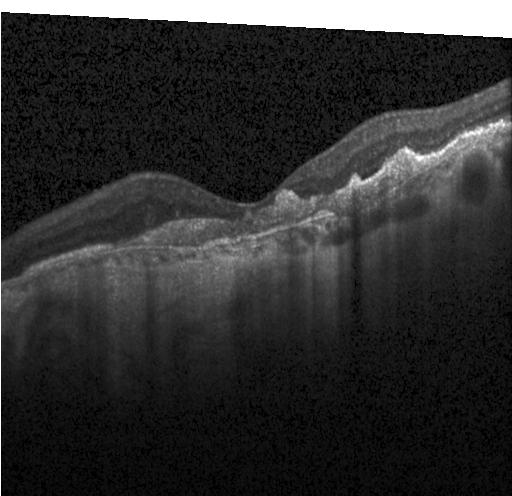

Impression: choroidal neovascularization (CNV).